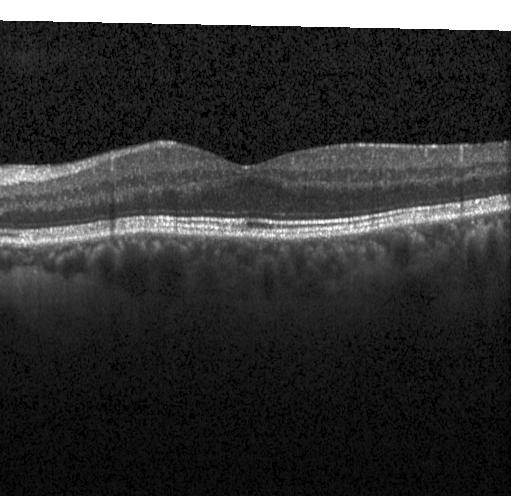
Neither choroidal neovascularization, diabetic macular edema, nor drusen.